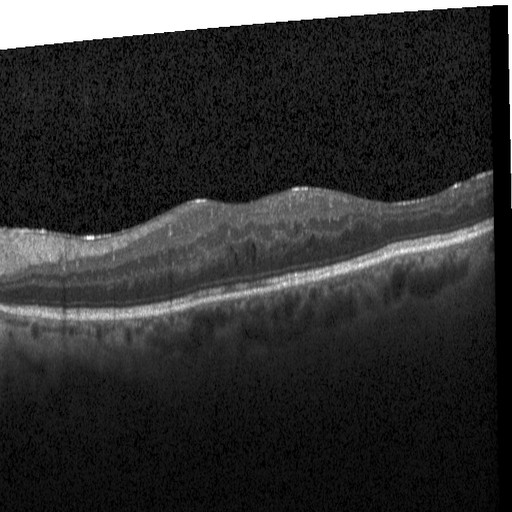 Retinal OCT B-scan · spectral-domain optical coherence tomography — Impression: diabetic macular edema (DME).